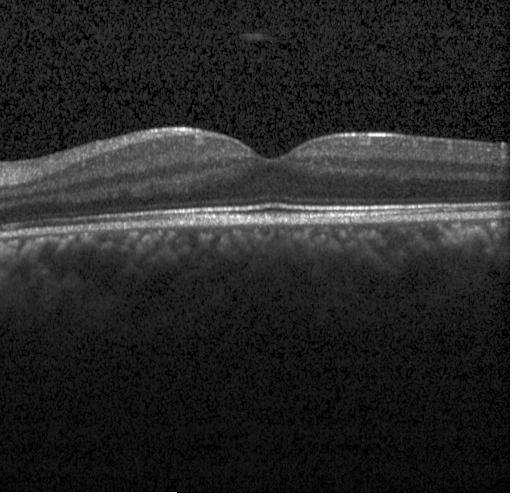 Dx: no choroidal neovascularization, diabetic macular edema, or drusen.